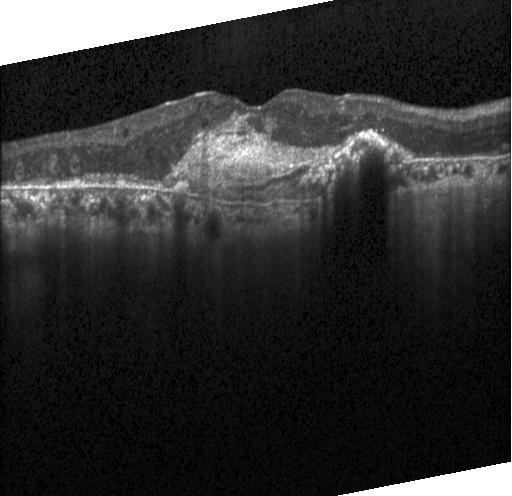

Impression: a choroidal neovascular membrane.